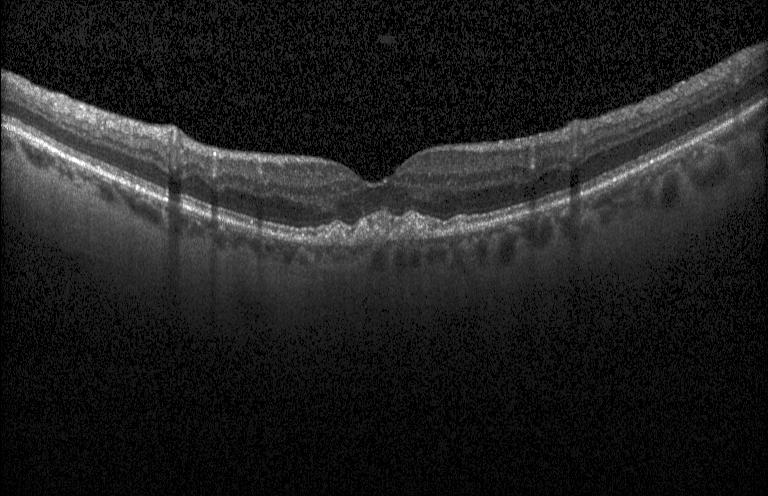

Through the macula; OCT line scan — Diagnosis: sub-RPE drusenoid deposits.